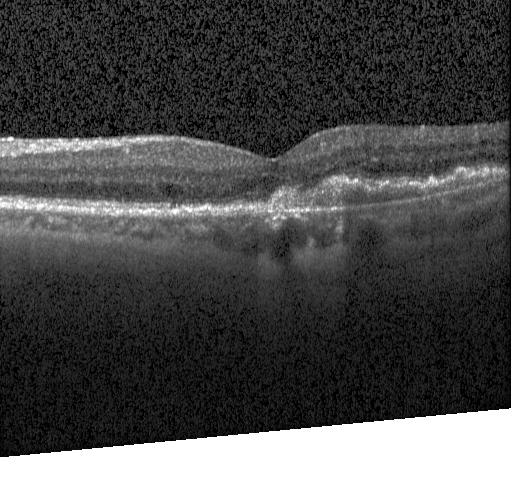 Retinal OCT cross-section.
OCT finding: a choroidal neovascular membrane.